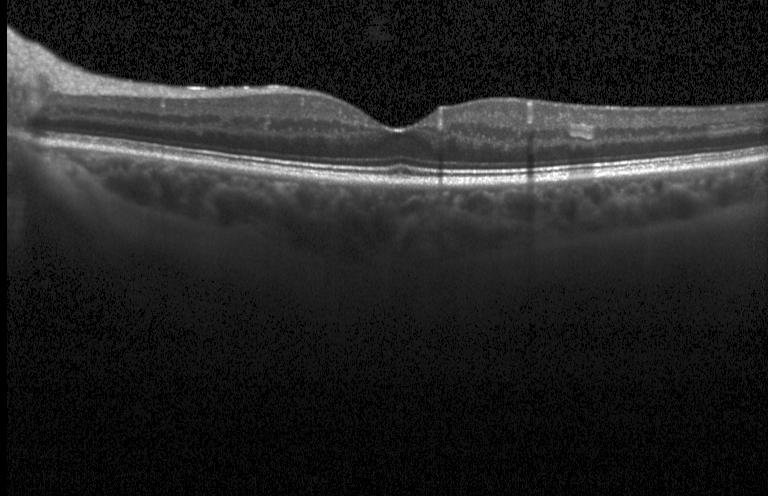

Optical coherence tomography scan. Finding: no CNV, DME, or drusen.